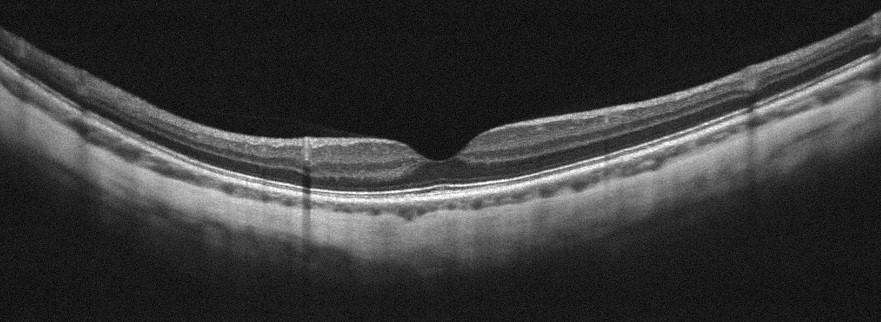 Instrument: Optovue Avanti RTVue XR; retinal OCT cross-section; through the macula. Impression: no AMD, DME, ERM, RAO, RVO, or VID.